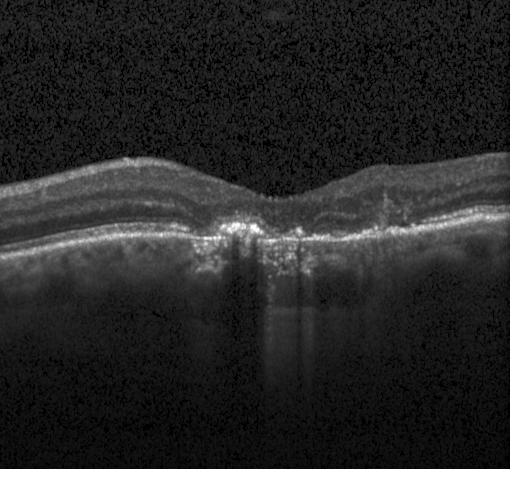

Horizontal scan through the fovea; optical coherence tomography B-scan
This B-scan demonstrates choroidal neovascularization.